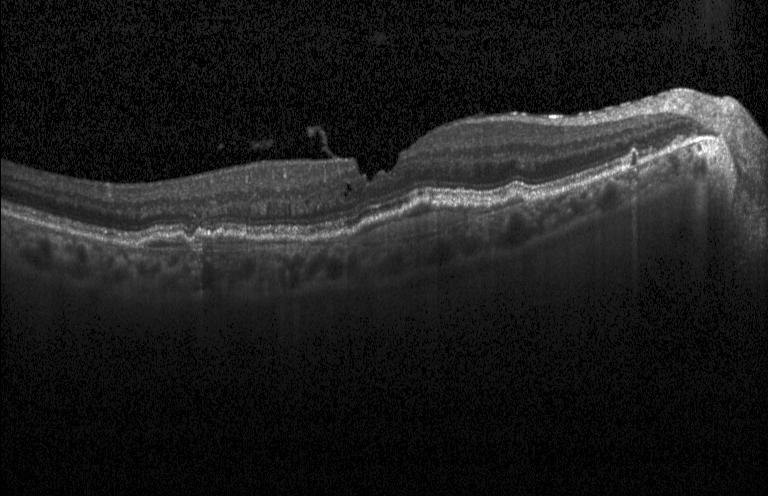

Dx: a choroidal neovascular membrane.